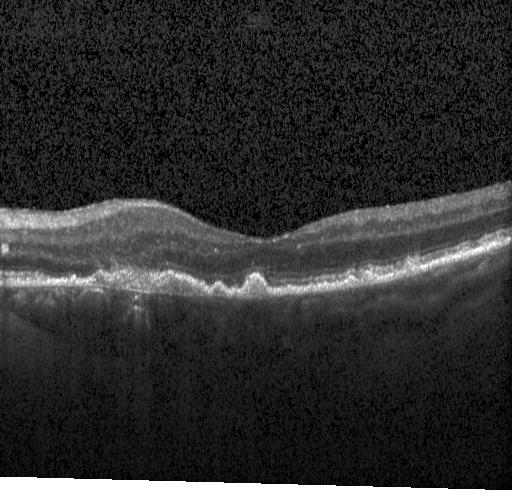 Spectral-domain optical coherence tomography; Heidelberg Spectralis; optical coherence tomography scan — The scan shows a choroidal neovascular membrane.